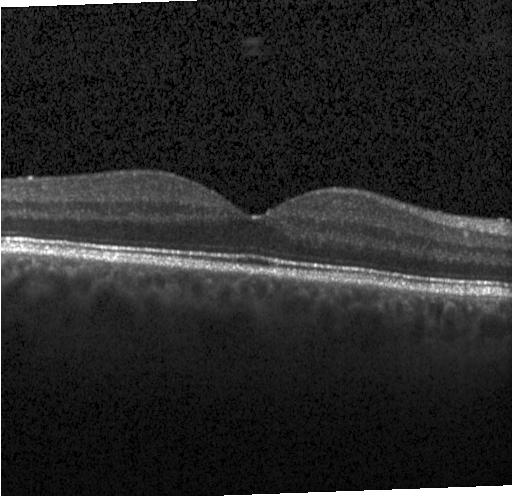
Impression: no choroidal neovascularization, no diabetic macular edema, and no drusen.